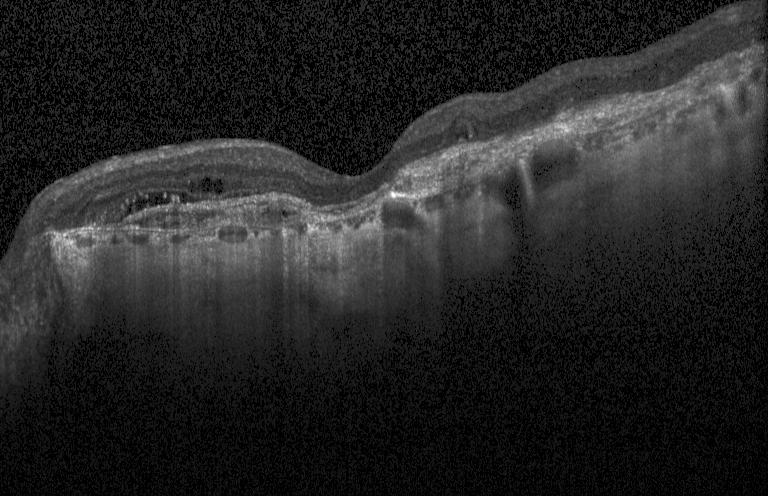
Macular scan. Acquired on a Heidelberg Spectralis. Spectral-domain optical coherence tomography. Retinal OCT B-scan. Finding: CNV.